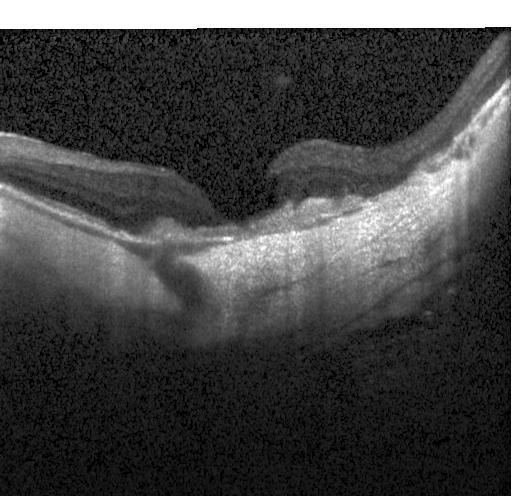
Diagnosis: a choroidal neovascular membrane.